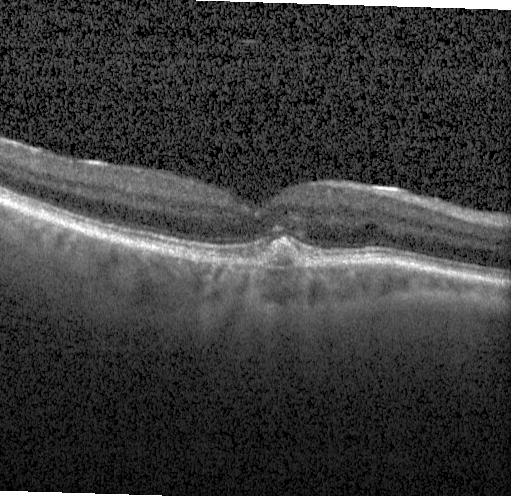 OCT scan showing a choroidal neovascular membrane.